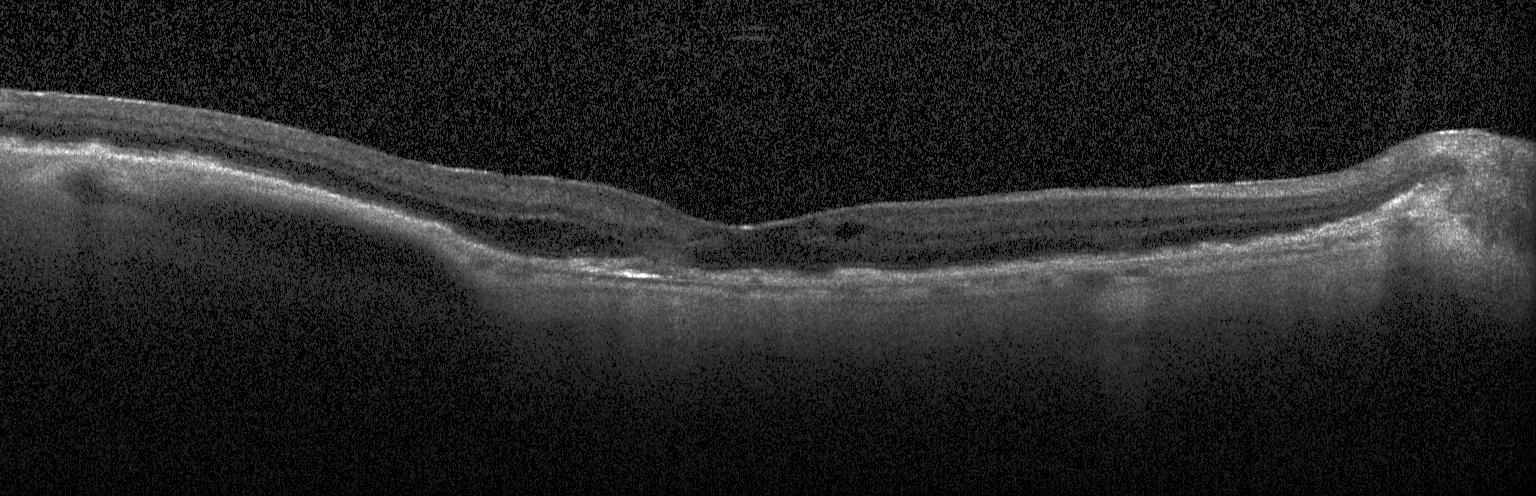
The scan shows choroidal neovascularization.